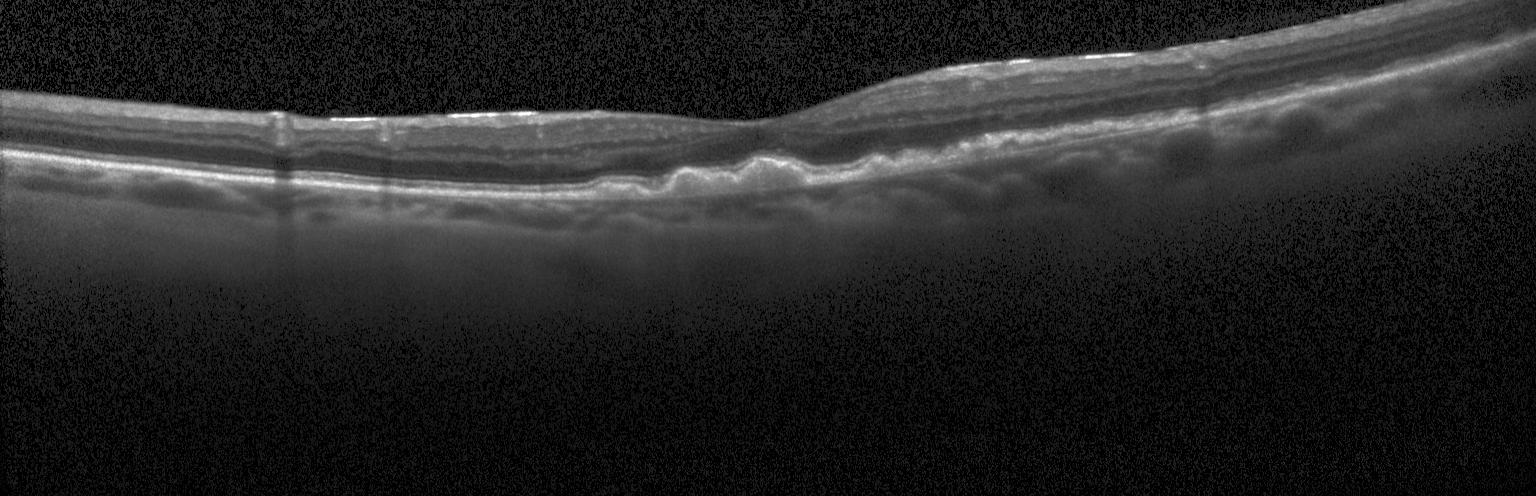
Retinal OCT B-scan.
The scan shows sub-RPE drusenoid deposits.